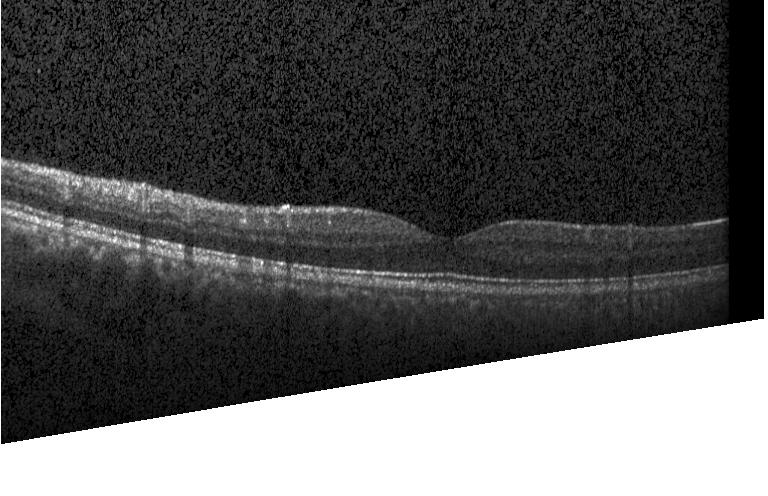

Diagnosis: no CNV, no DME, and no drusen.